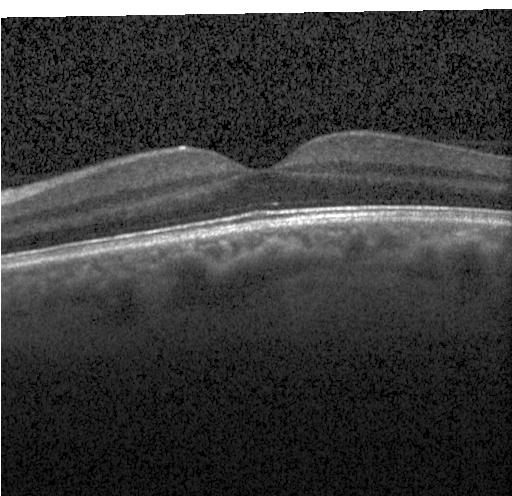 Spectral-domain OCT, retinal OCT B-scan — Impression: neither choroidal neovascularization, diabetic macular edema, nor drusen.